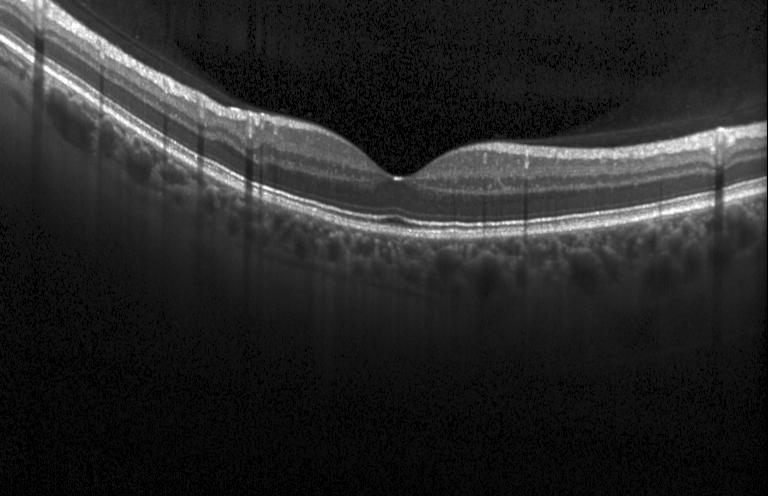 OCT line scan · acquired on a Heidelberg Spectralis — Dx: neither CNV, DME, nor drusen.